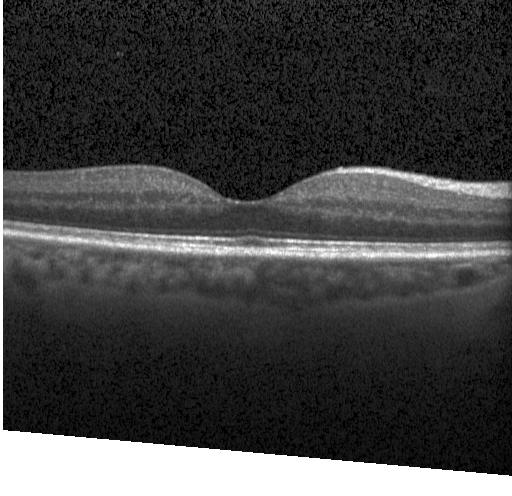 OCT line scan
This B-scan demonstrates neither CNV, DME, nor drusen.